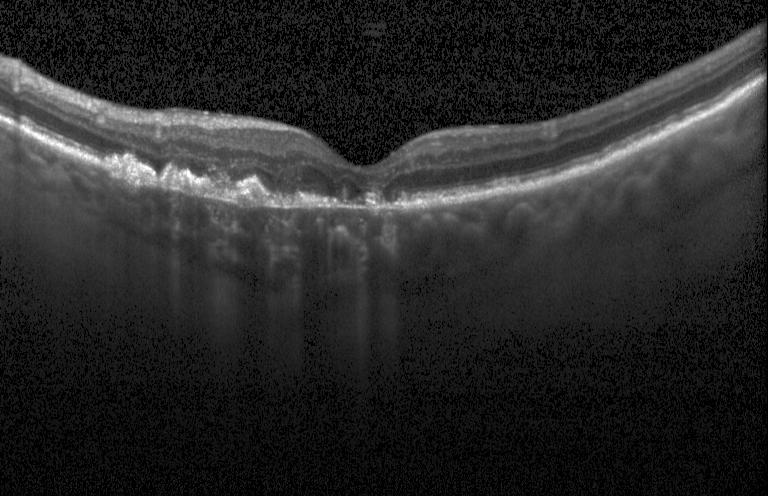
SD-OCT, centered on the fovea, OCT line scan, instrument: Heidelberg Spectralis. Finding: a choroidal neovascular membrane.